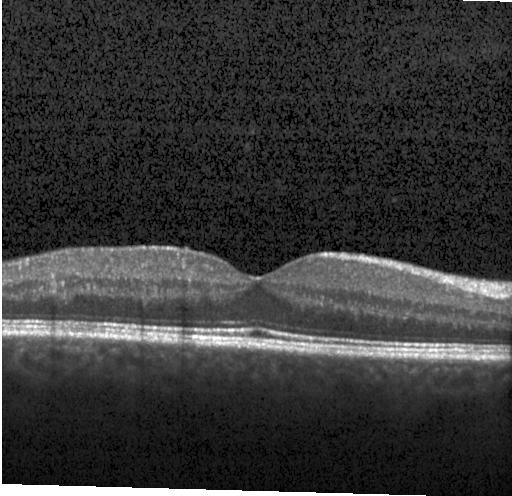
OCT B-scan showing no evidence of choroidal neovascularization, diabetic macular edema, or drusen.